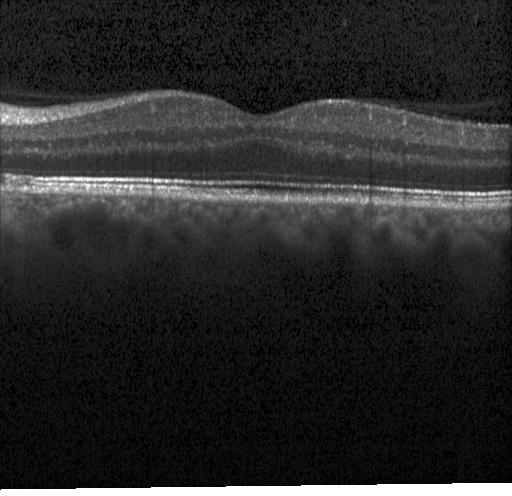

Neither choroidal neovascularization, diabetic macular edema, nor drusen.